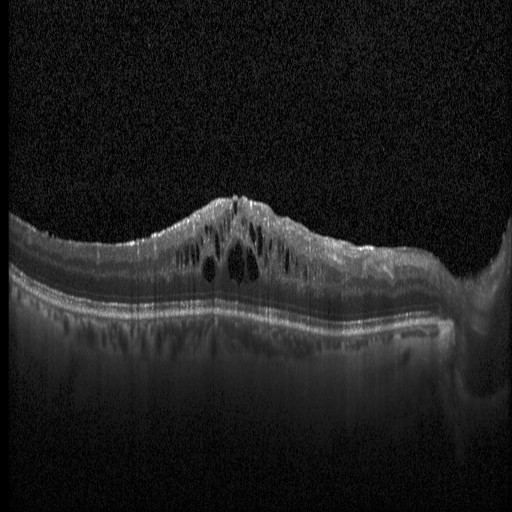
Horizontal scan through the fovea, optical coherence tomography B-scan, Heidelberg Spectralis. Diabetic macular edema (DME).